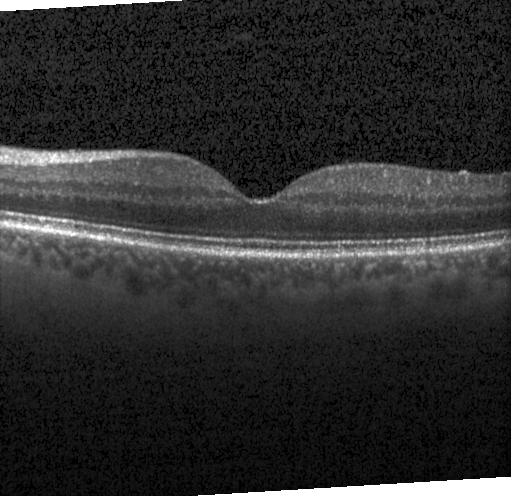 OCT B-scan; spectral-domain optical coherence tomography.
Finding: neither CNV, DME, nor drusen.